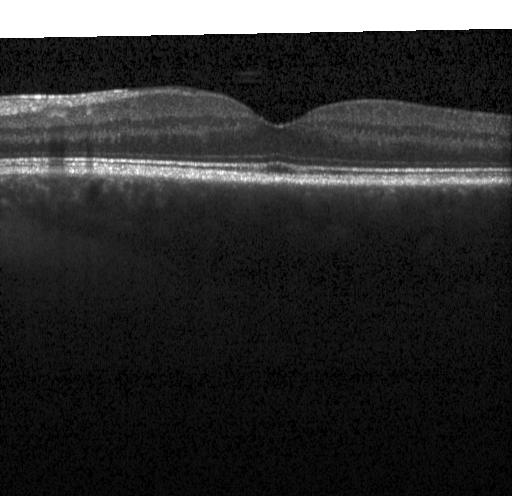 OCT B-scan showing no evidence of CNV, DME, or drusen.